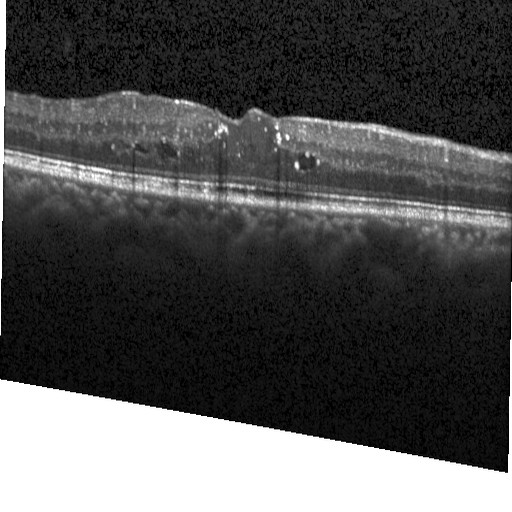 OCT finding: diabetic macular edema (DME).